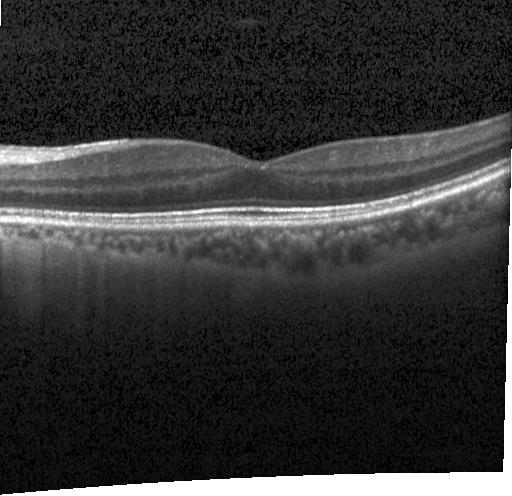

Heidelberg Spectralis OCT system, retinal OCT cross-section, fovea-centered, SD-OCT.
Assessment: no evidence of choroidal neovascularization, diabetic macular edema, or drusen.